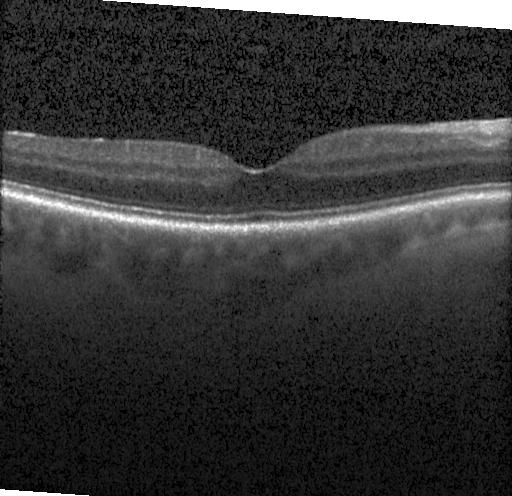 OCT B-scan. SD-OCT. Fovea-centered. Acquired on a Heidelberg Spectralis — Diagnosis: no evidence of choroidal neovascularization, diabetic macular edema, or drusen.